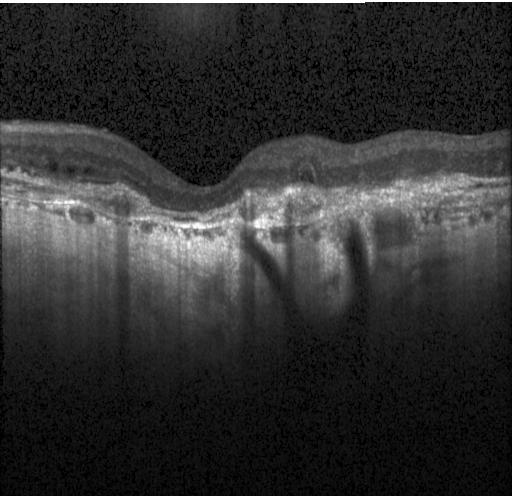 Instrument: Heidelberg Spectralis; OCT line scan. Finding: a choroidal neovascular membrane.